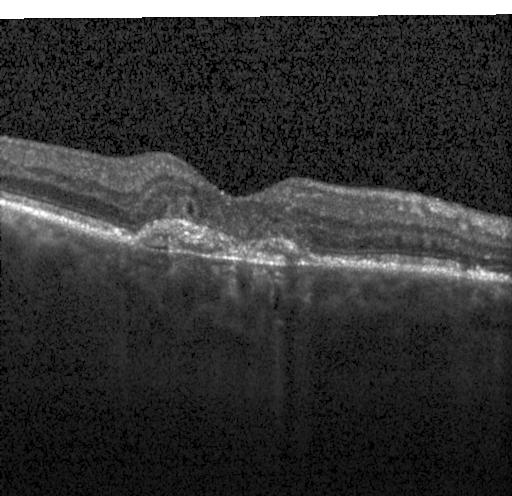

Impression: a choroidal neovascular membrane.